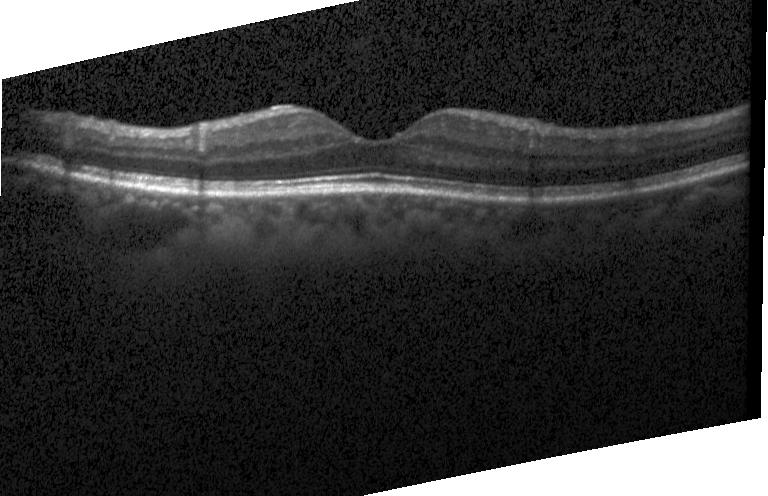
Retinal OCT cross-section — Macular OCT: no choroidal neovascularization, diabetic macular edema, or drusen.